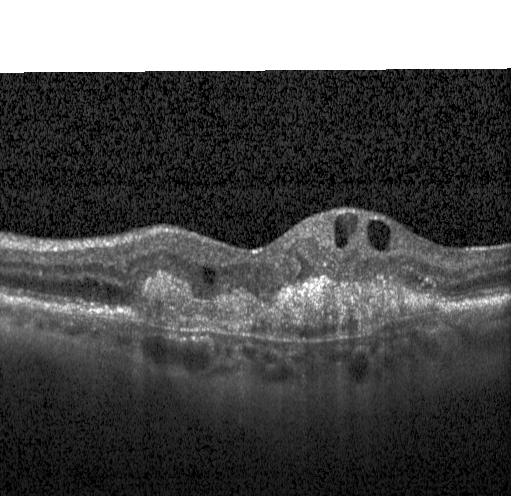 OCT finding: a choroidal neovascular membrane.